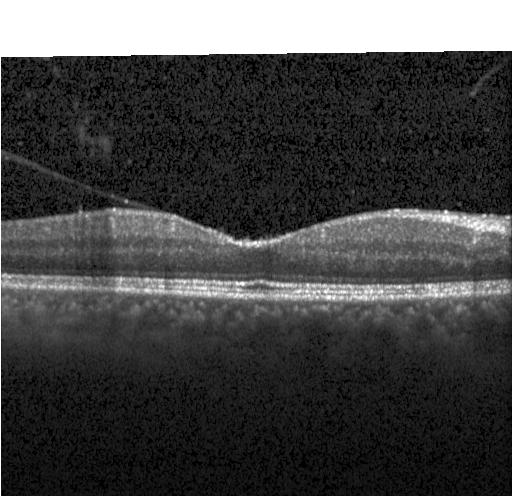
Horizontal scan through the fovea · optical coherence tomography B-scan.
OCT finding: no choroidal neovascularization, no diabetic macular edema, and no drusen.